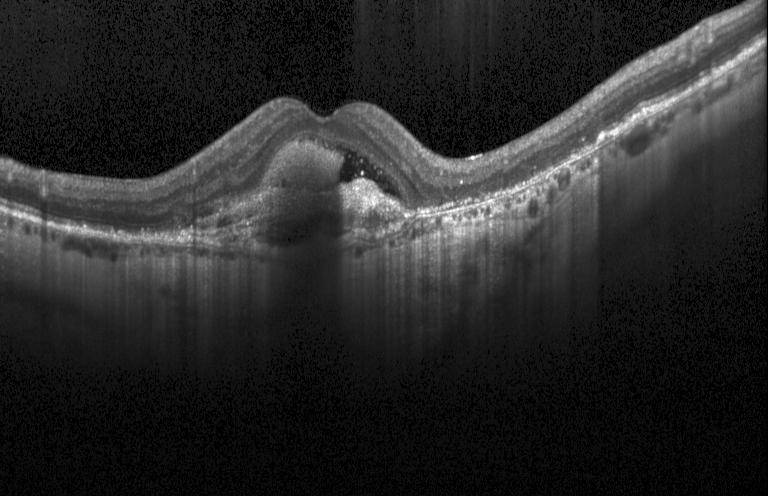 Retinal OCT cross-section, spectral-domain OCT. Impression: a choroidal neovascular membrane.